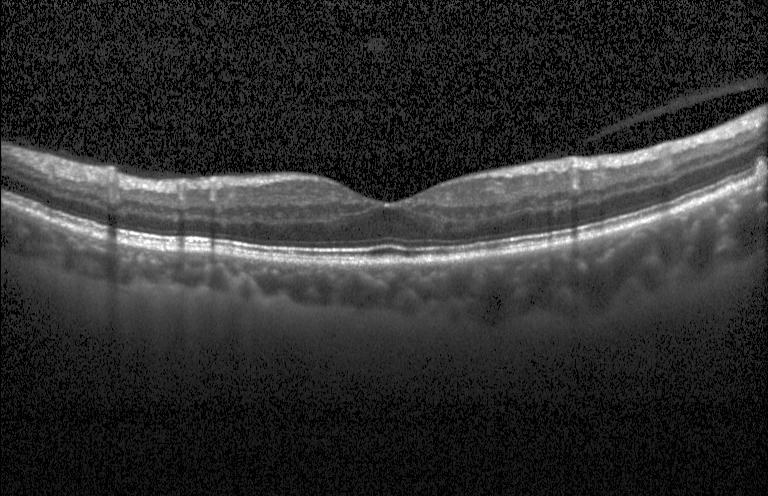

OCT B-scan
No choroidal neovascularization, no diabetic macular edema, and no drusen.